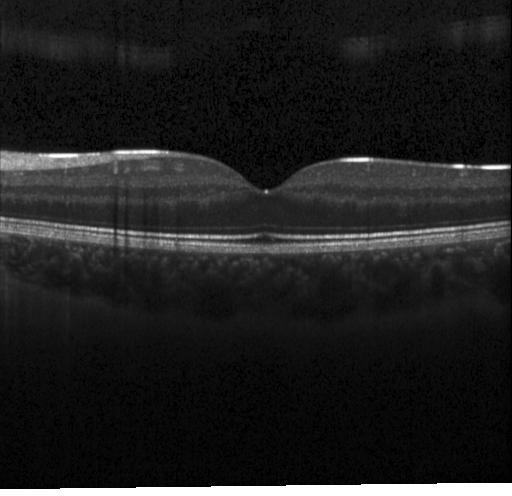 The scan shows neither choroidal neovascularization, diabetic macular edema, nor drusen.